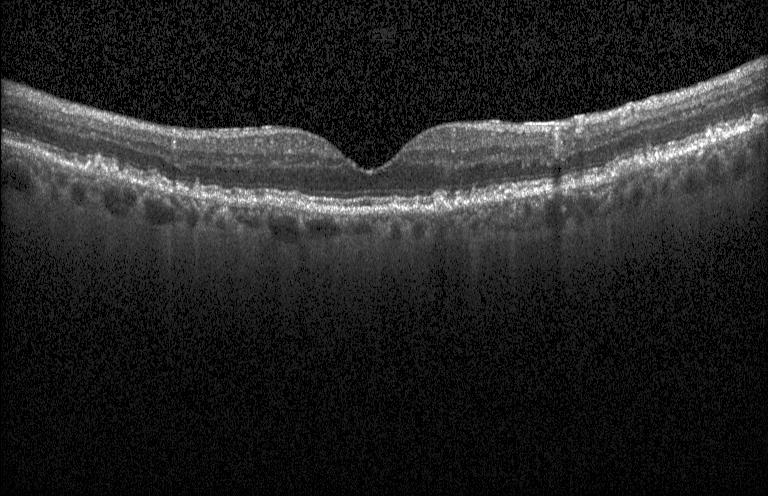

OCT line scan. Acquired on a Heidelberg Spectralis
This B-scan demonstrates drusen.